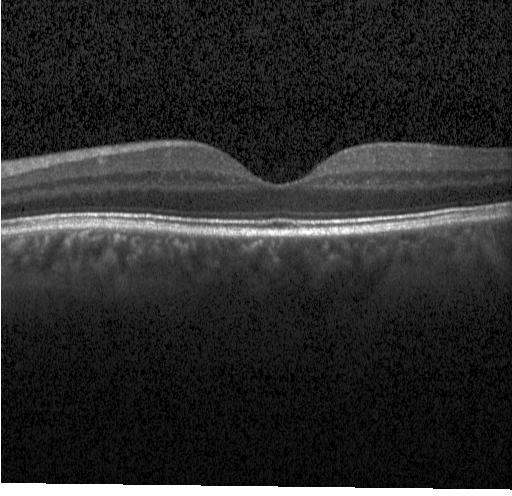

This B-scan demonstrates no choroidal neovascularization, diabetic macular edema, or drusen.